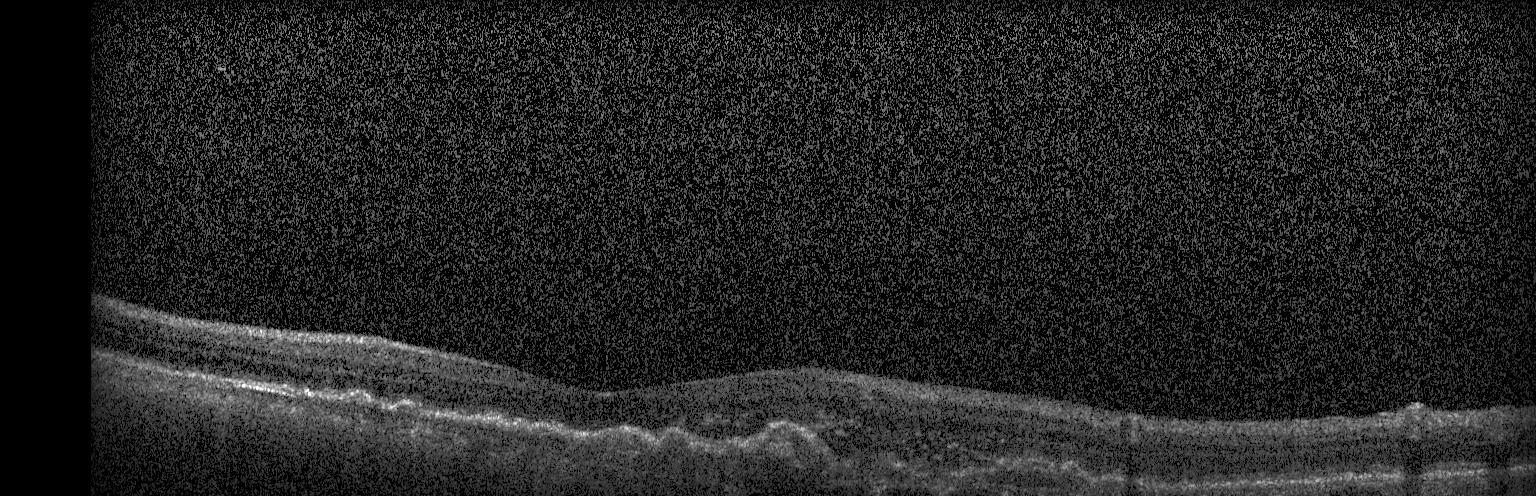 Retinal OCT cross-section. Heidelberg Spectralis. Choroidal neovascularization (CNV).